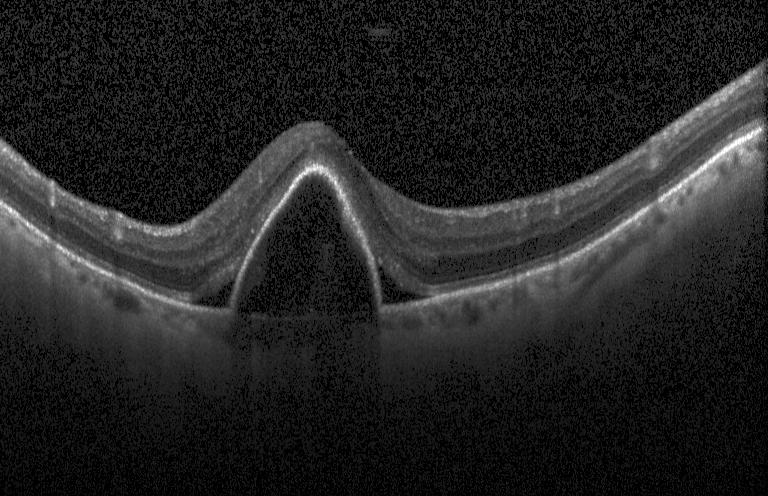

Instrument: Heidelberg Spectralis · centered on the fovea · OCT line scan.
Diagnosis: a choroidal neovascular membrane.